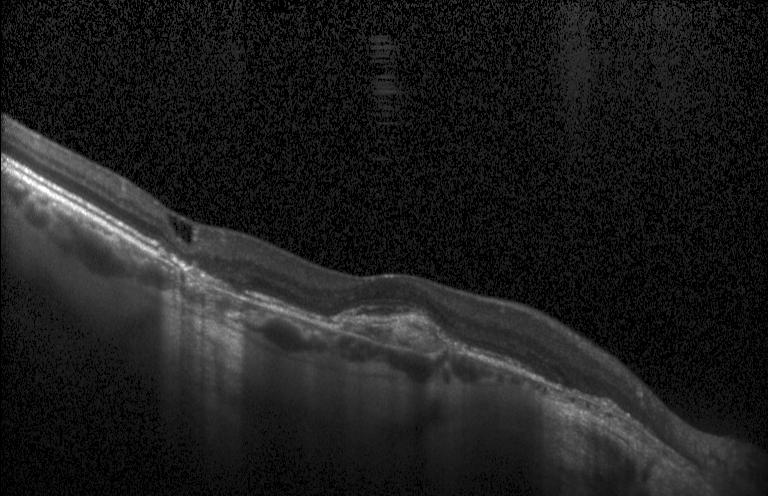 OCT B-scan showing choroidal neovascularization (CNV).